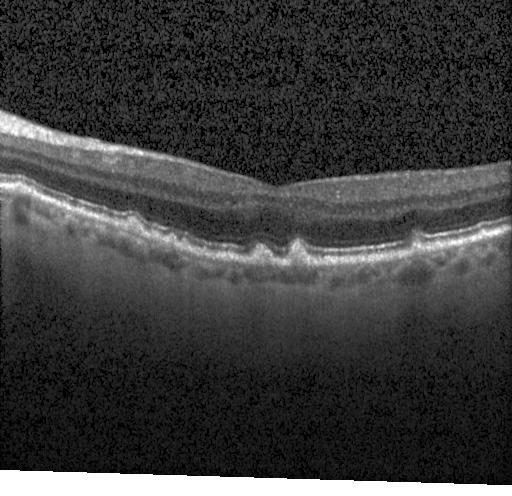
Drusen.